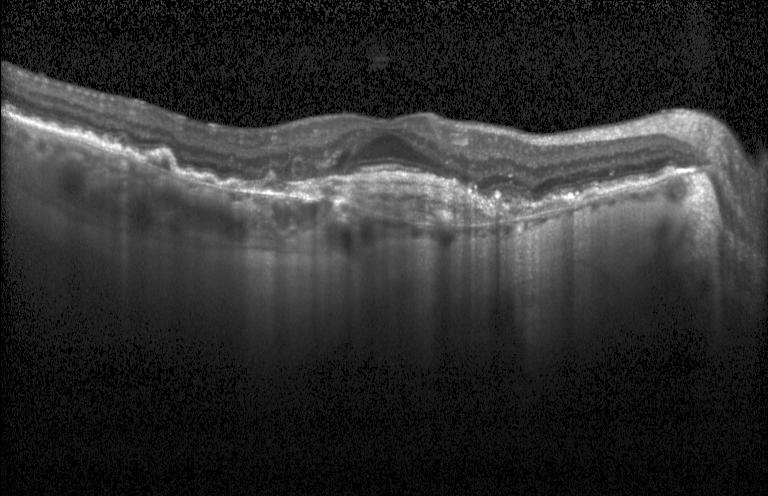
Finding: CNV.